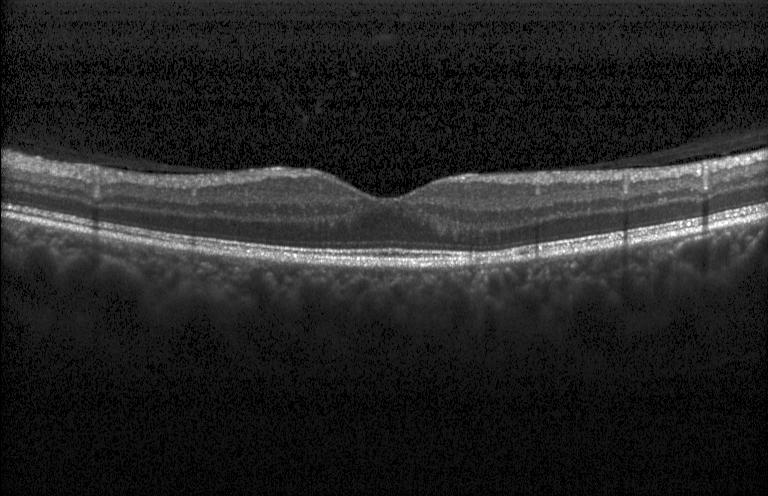
Acquired on a Heidelberg Spectralis, OCT B-scan
Assessment: no choroidal neovascularization, no diabetic macular edema, and no drusen.